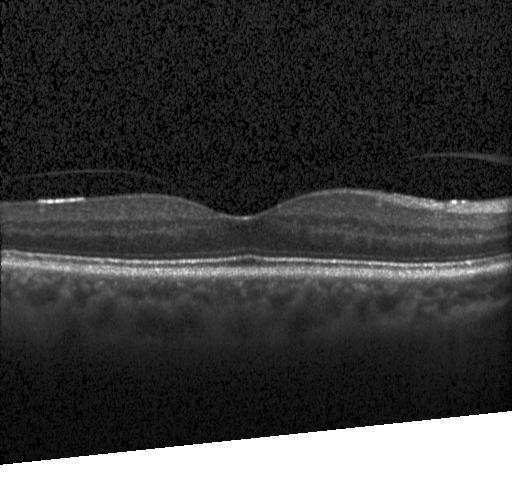

OCT scan showing no evidence of choroidal neovascularization, diabetic macular edema, or drusen.